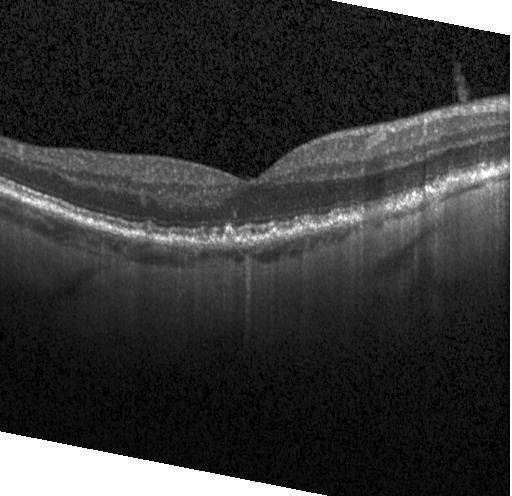

Spectral-domain OCT; acquired on a Heidelberg Spectralis; fovea-centered; OCT line scan.
Dx: multiple drusen.